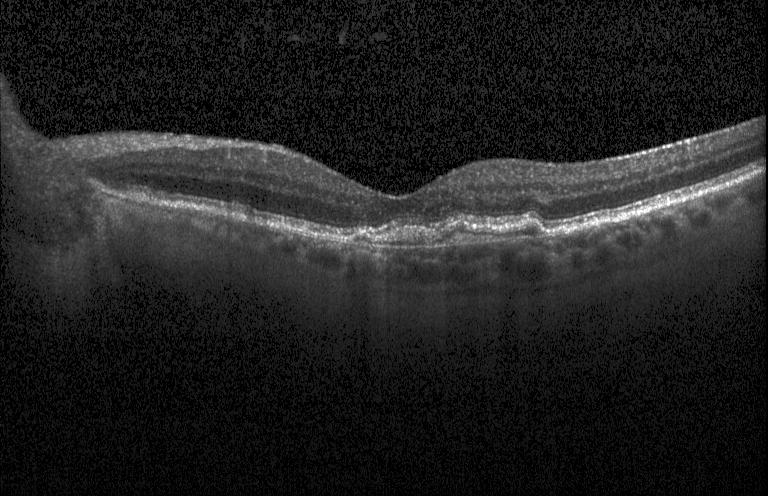

Dx: a choroidal neovascular membrane.